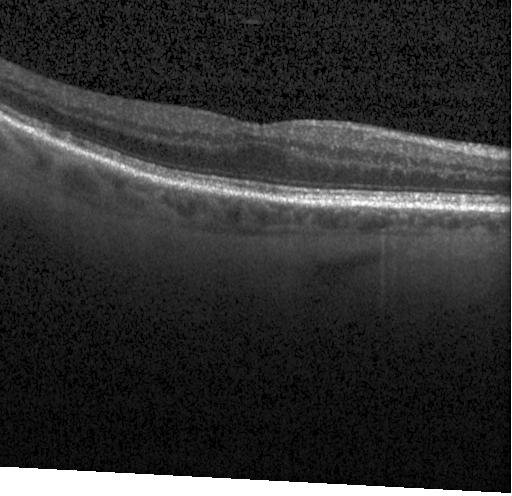
Impression: neither choroidal neovascularization, diabetic macular edema, nor drusen.